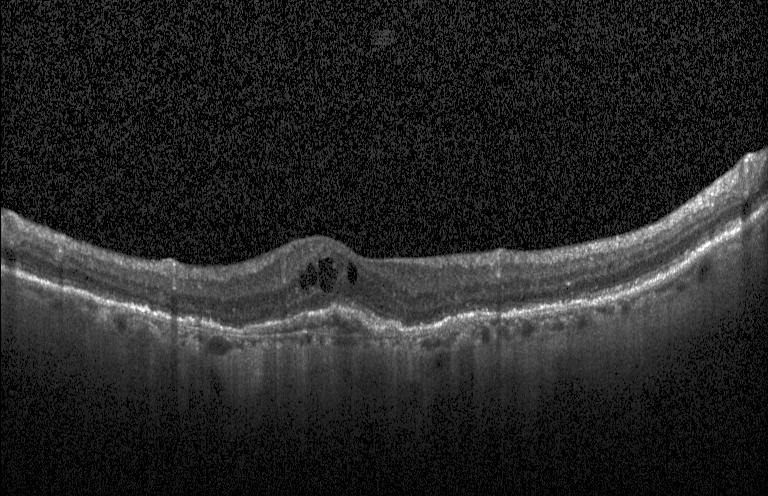

Through the macula; retinal OCT B-scan; Heidelberg Spectralis OCT system; SD-OCT
Finding: CNV.